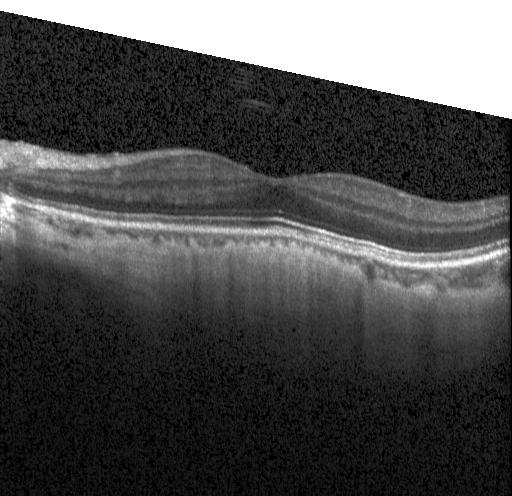 Macular scan. Retinal OCT cross-section.
Finding: neither choroidal neovascularization, diabetic macular edema, nor drusen.